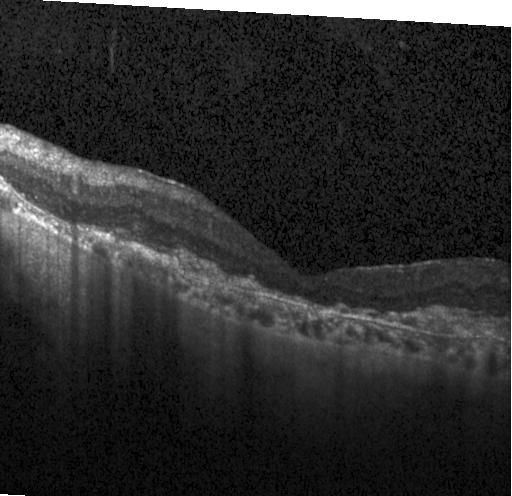 Choroidal neovascularization.